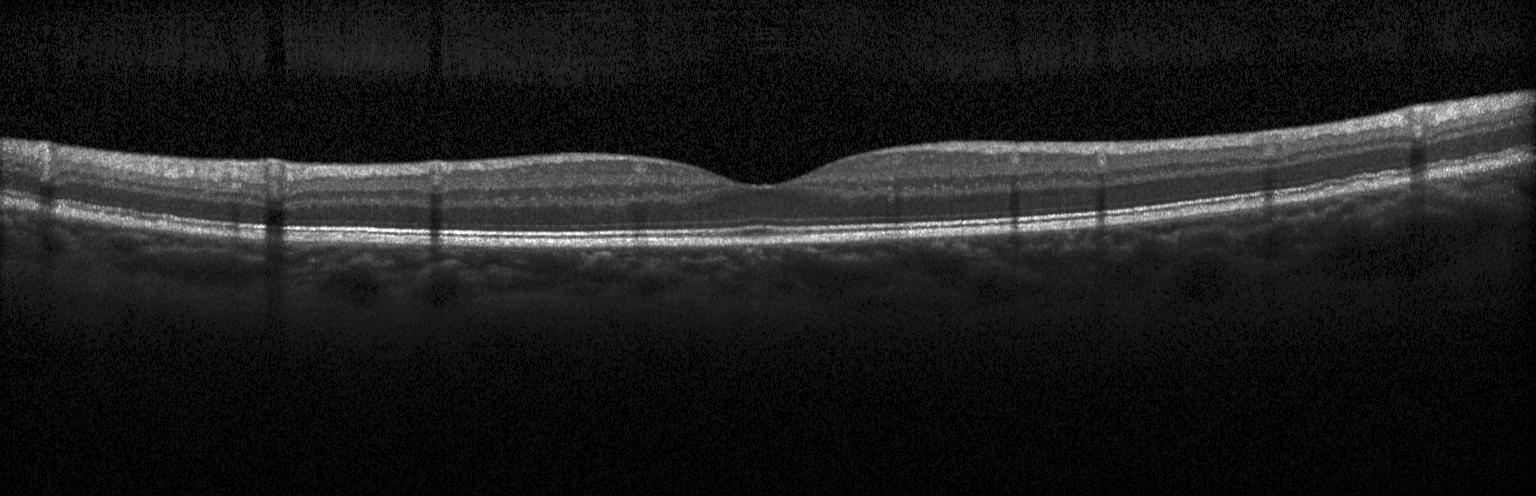 Optical coherence tomography B-scan. Macular OCT: no choroidal neovascularization, no diabetic macular edema, and no drusen.